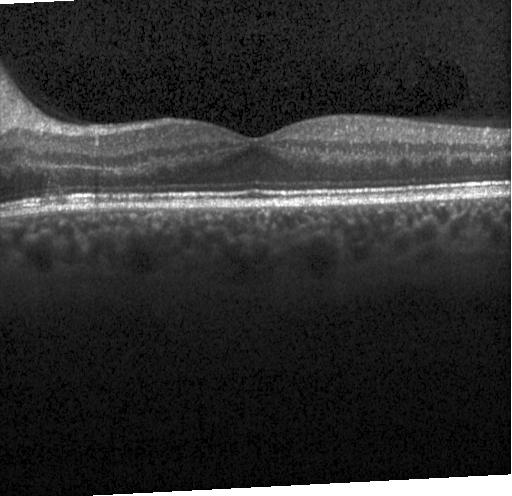 Optical coherence tomography scan — Macular OCT: no evidence of CNV, DME, or drusen.